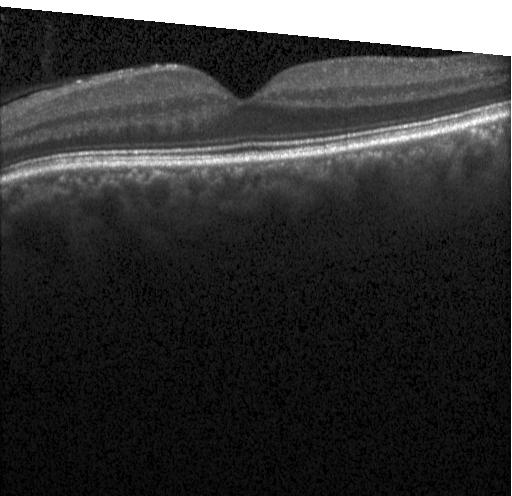
OCT line scan. Centered on the fovea. Acquired on a Heidelberg Spectralis. SD-OCT
Impression: no choroidal neovascularization, no diabetic macular edema, and no drusen.